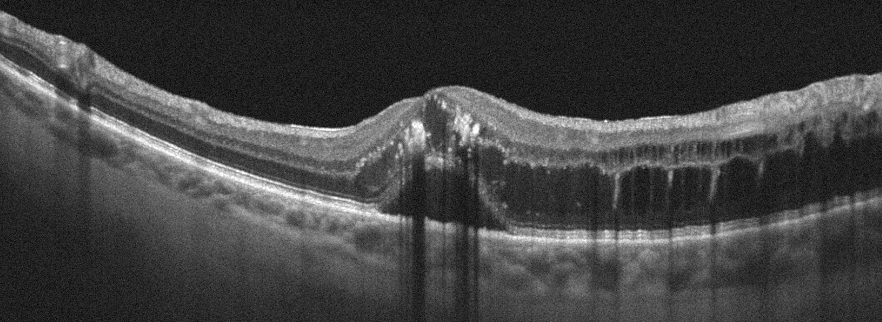 OCT B-scan — The scan shows retinal vein occlusion.